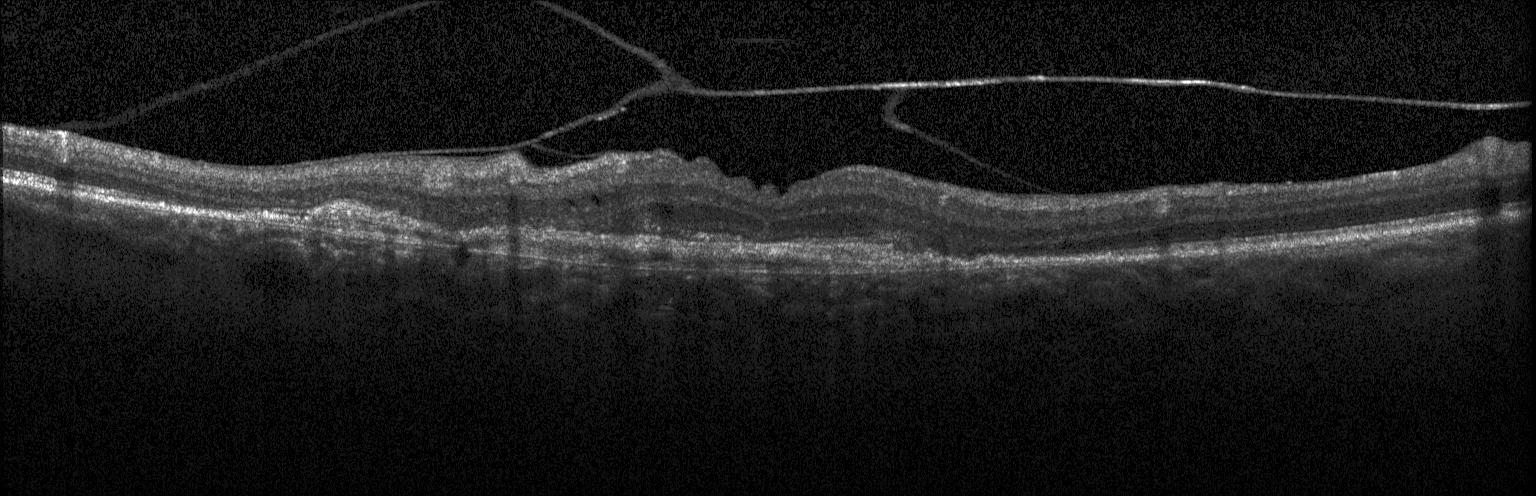 Macular scan; retinal OCT cross-section; Heidelberg Spectralis; spectral-domain optical coherence tomography.
Dx: a choroidal neovascular membrane.